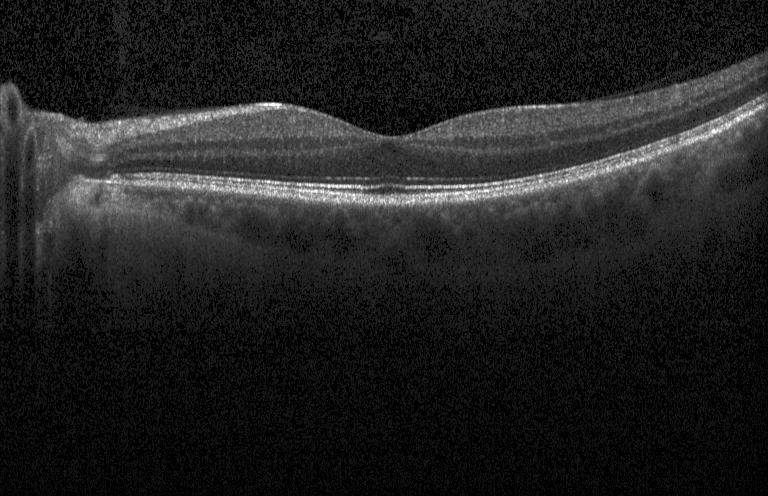
Finding: no evidence of choroidal neovascularization, diabetic macular edema, or drusen.